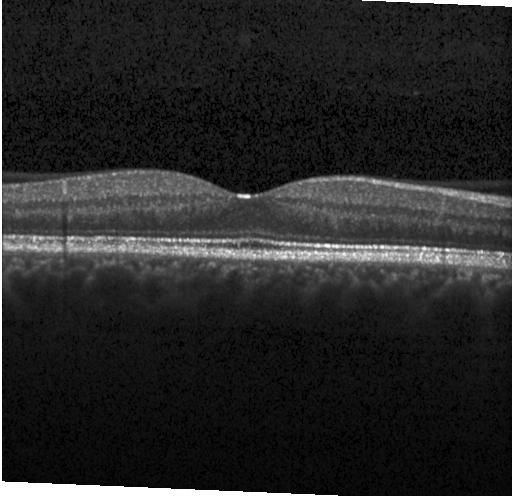

Optical coherence tomography scan, fovea-centered. Finding: no evidence of choroidal neovascularization, diabetic macular edema, or drusen.